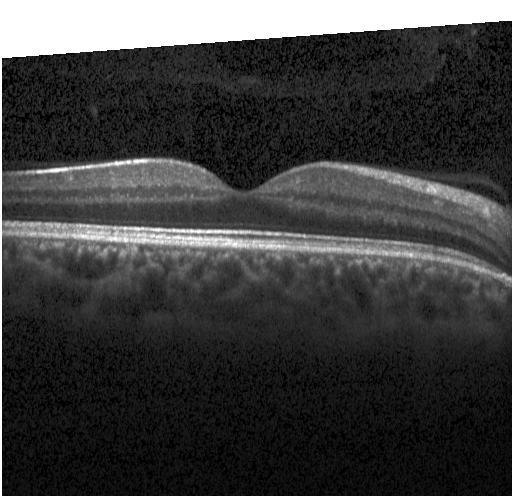
Assessment: no CNV, DME, or drusen.